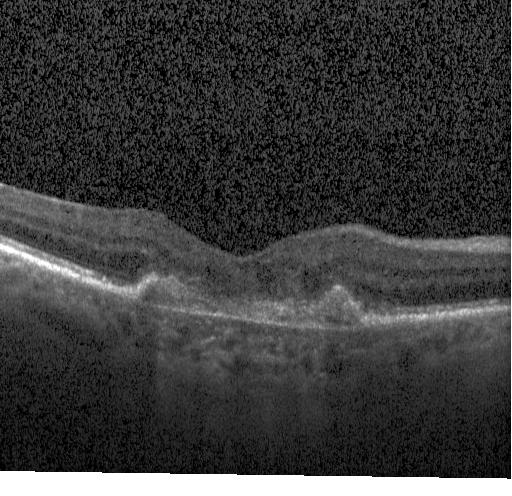 OCT line scan. Spectral-domain OCT. Centered on the fovea. Heidelberg Spectralis — Assessment: a choroidal neovascular membrane.